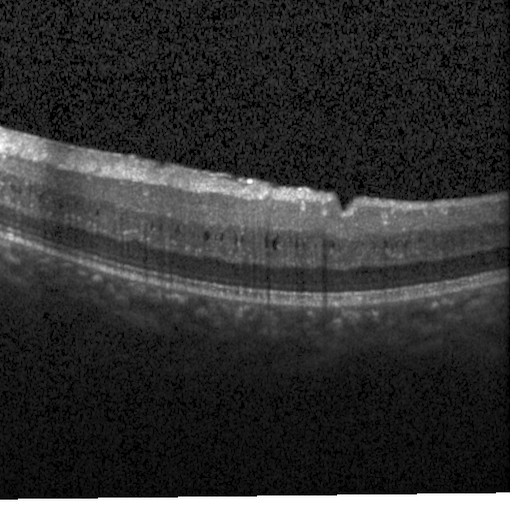 OCT line scan — Diagnosis: diabetic macular edema.